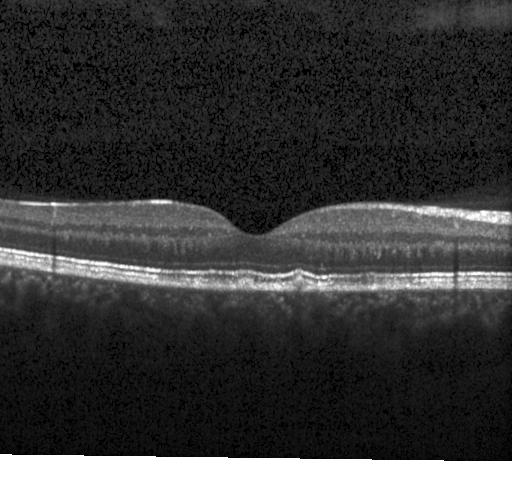
Optical coherence tomography scan; Heidelberg Spectralis; centered on the fovea; spectral-domain OCT — Diagnosis: sub-RPE drusenoid deposits.